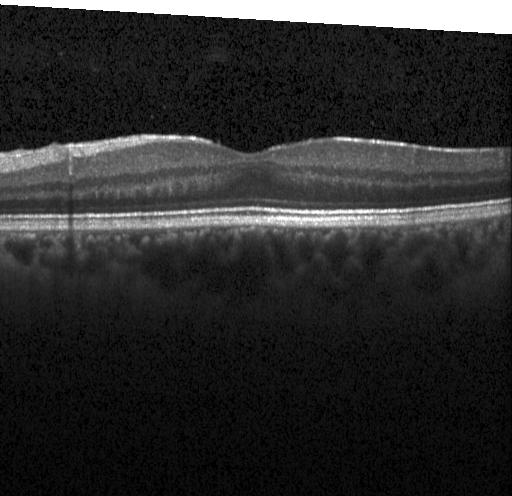

Optical coherence tomography scan · horizontal scan through the fovea. Diagnosis: no CNV, DME, or drusen.